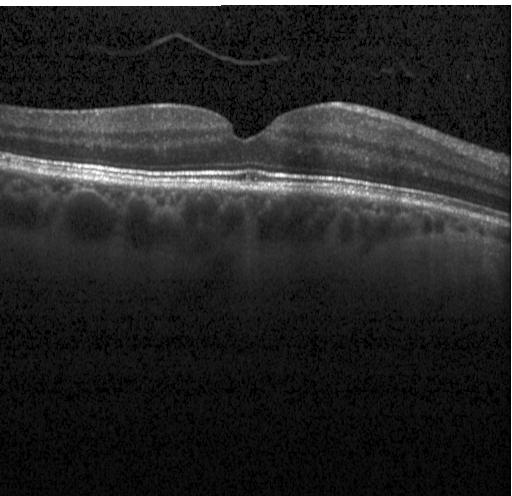

Macular OCT: neither choroidal neovascularization, diabetic macular edema, nor drusen.